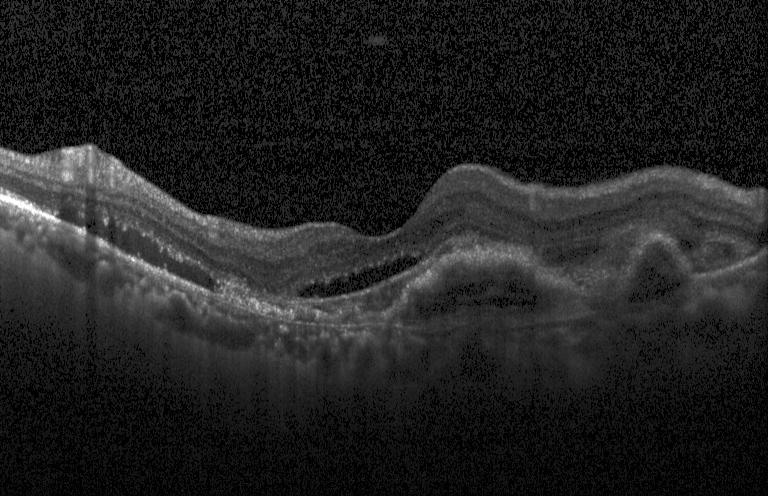 Retinal OCT B-scan.
Diagnosis: CNV.